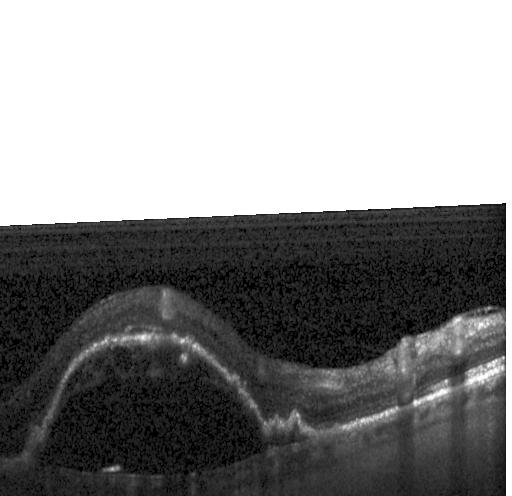

Heidelberg Spectralis OCT system. Retinal OCT B-scan
Impression: choroidal neovascularization.